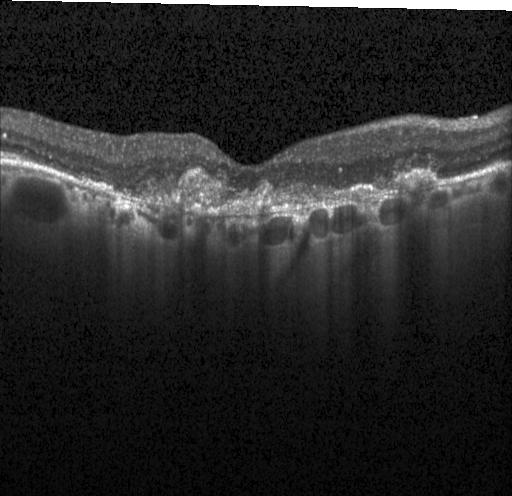

OCT finding: a choroidal neovascular membrane.